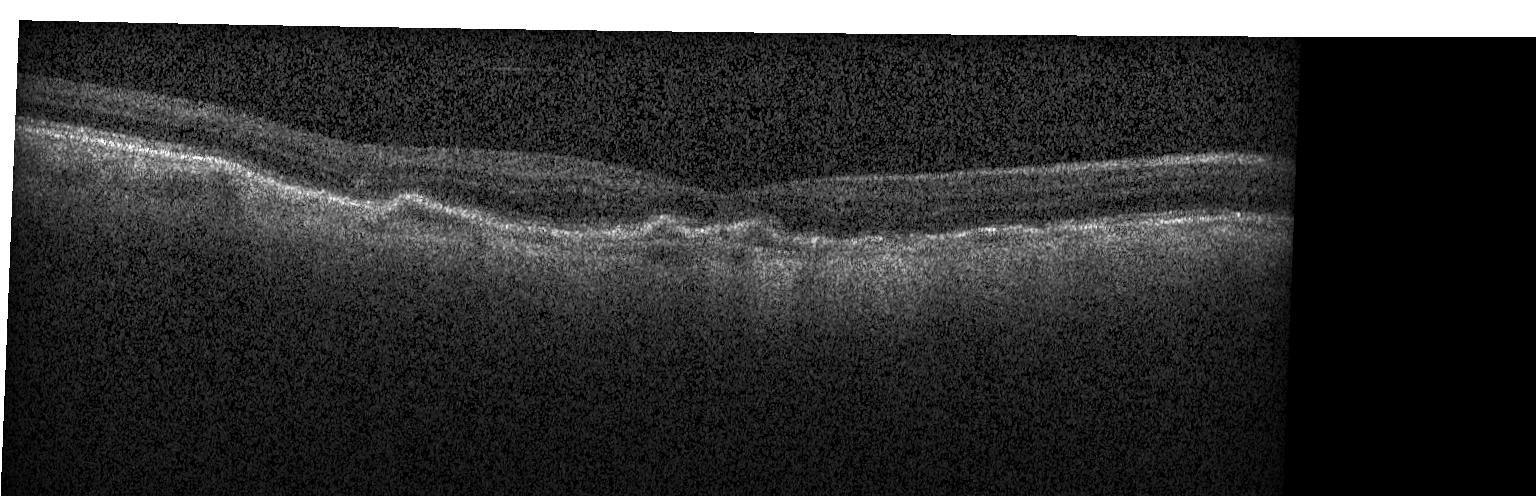
Finding: a choroidal neovascular membrane.